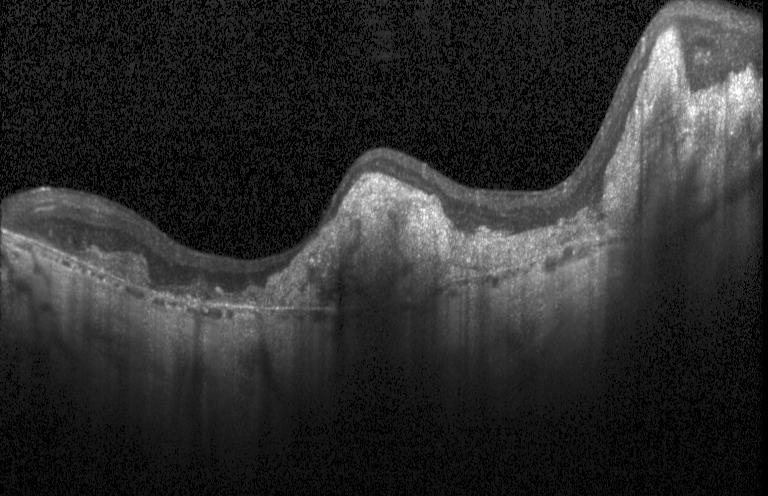
This B-scan demonstrates a choroidal neovascular membrane.